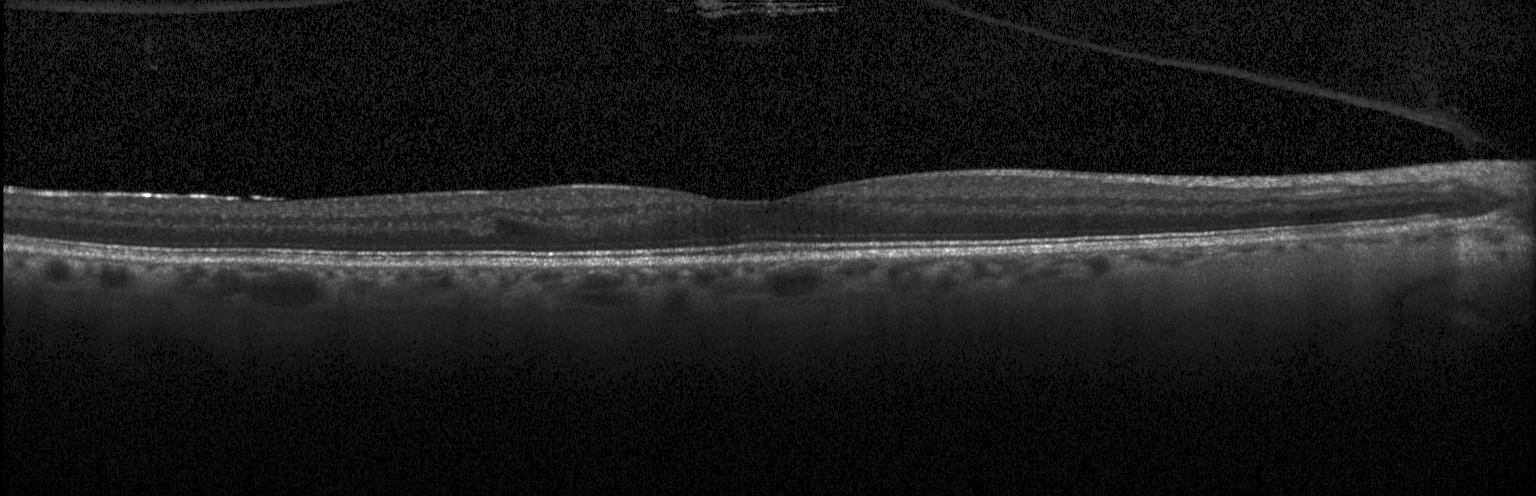
Heidelberg Spectralis; OCT line scan.
The scan shows no evidence of choroidal neovascularization, diabetic macular edema, or drusen.